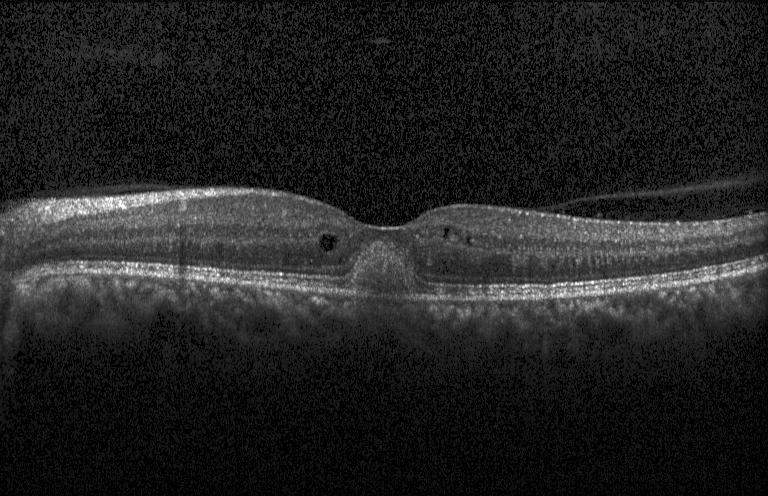

Optical coherence tomography scan
Dx: choroidal neovascularization (CNV).